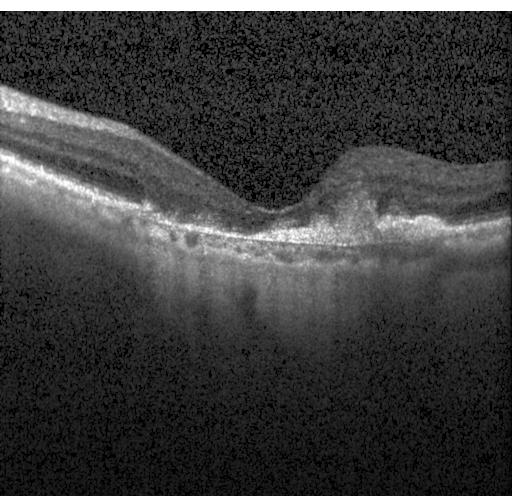

Fovea-centered. OCT line scan. Instrument: Heidelberg Spectralis. Spectral-domain OCT. Finding: choroidal neovascularization.